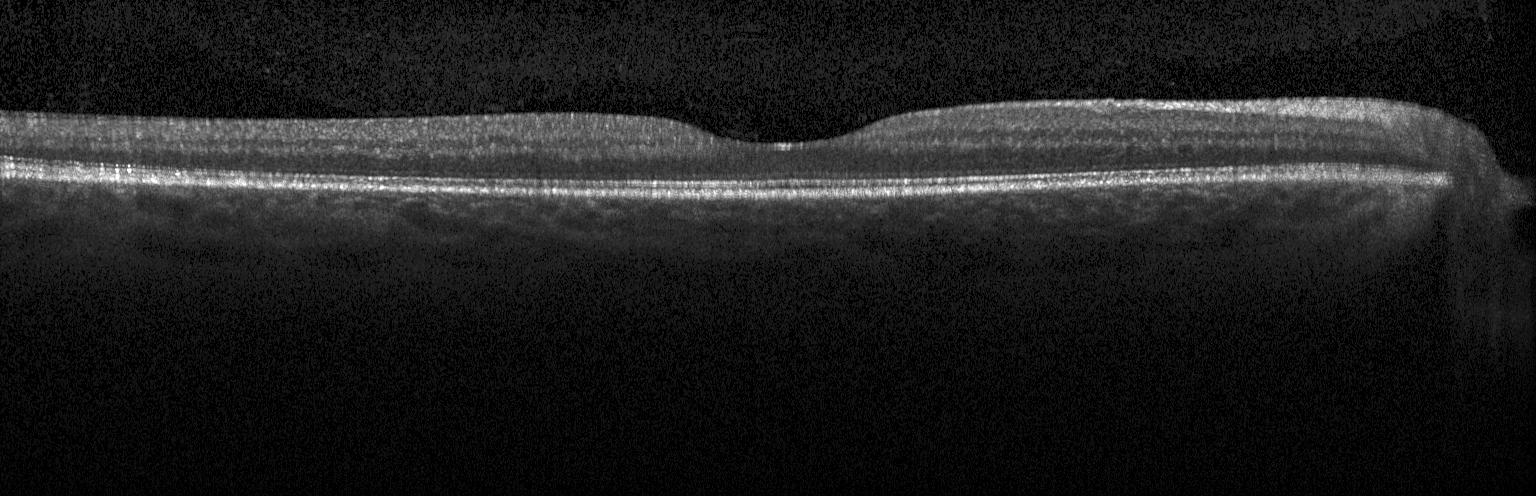
Retinal OCT B-scan. Finding: no choroidal neovascularization, diabetic macular edema, or drusen.